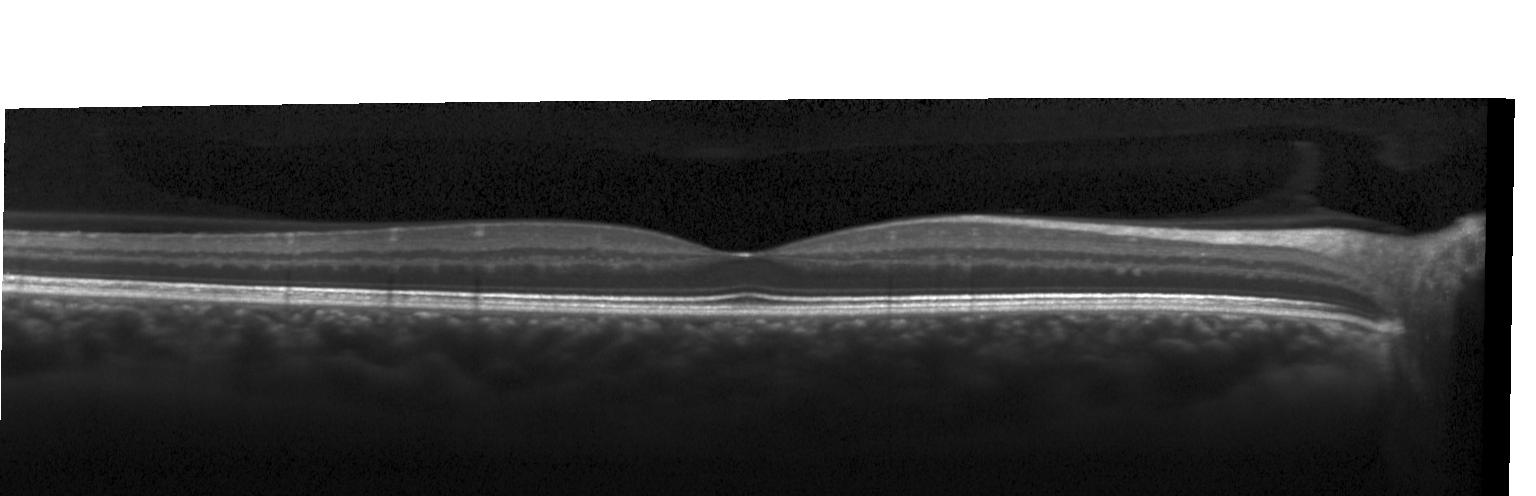 Retinal OCT cross-section — No evidence of CNV, DME, or drusen.